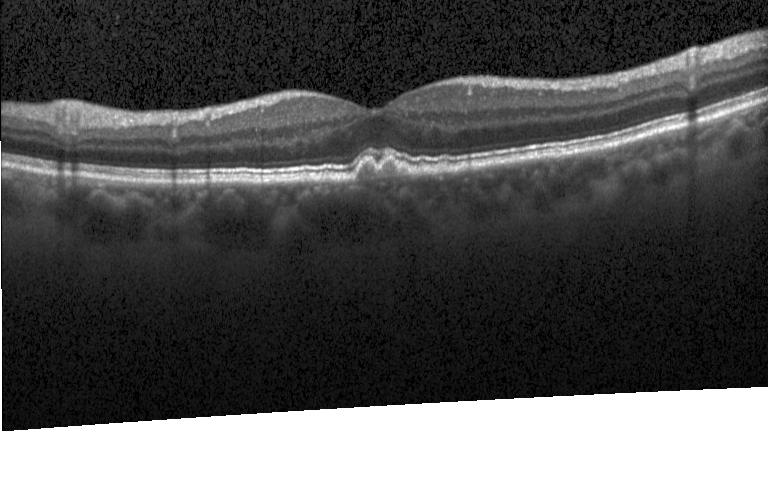
Dx: multiple drusen.